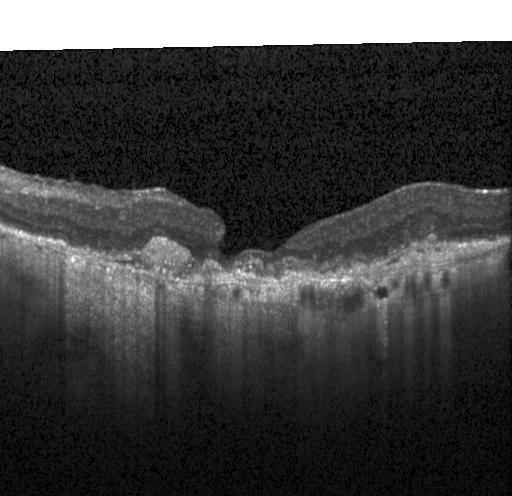 Diagnosis: a choroidal neovascular membrane.